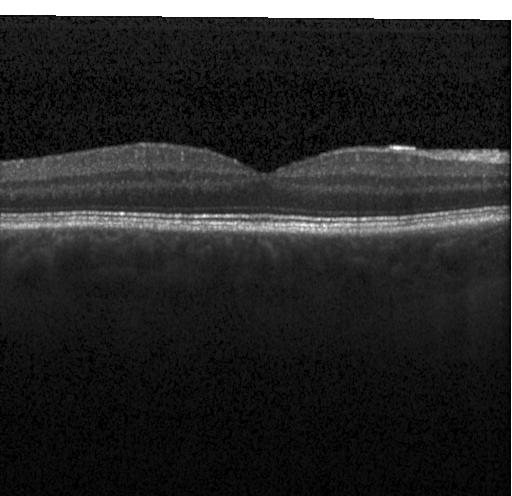
Spectral-domain OCT B-scan: no evidence of CNV, DME, or drusen.